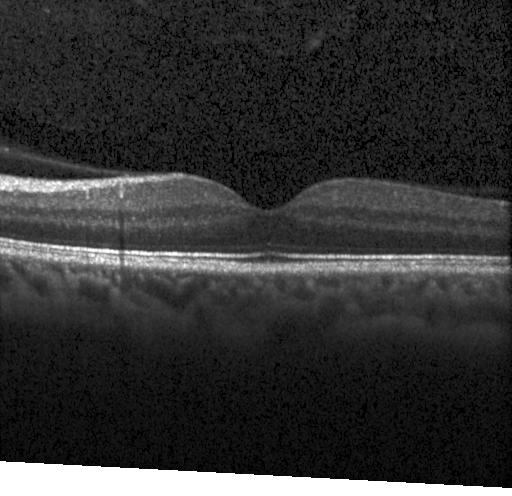

Retinal OCT B-scan · acquired on a Heidelberg Spectralis · SD-OCT · centered on the fovea — The scan shows no CNV, no DME, and no drusen.